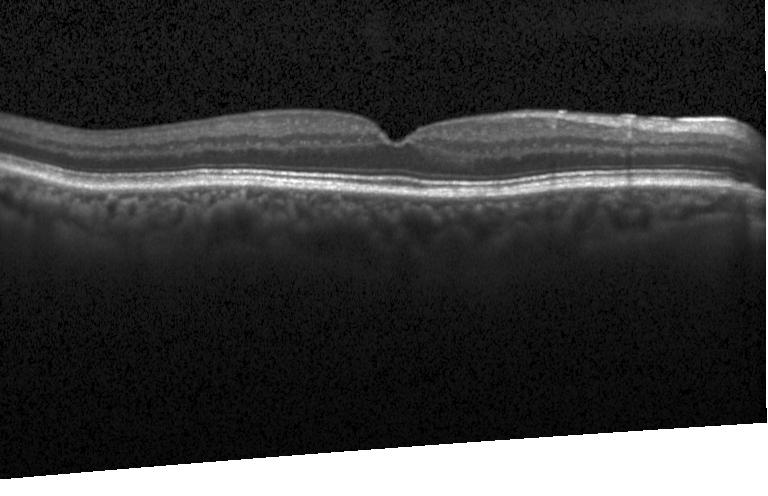

Optical coherence tomography B-scan. Acquired on a Heidelberg Spectralis. Spectral-domain OCT
The scan shows neither CNV, DME, nor drusen.